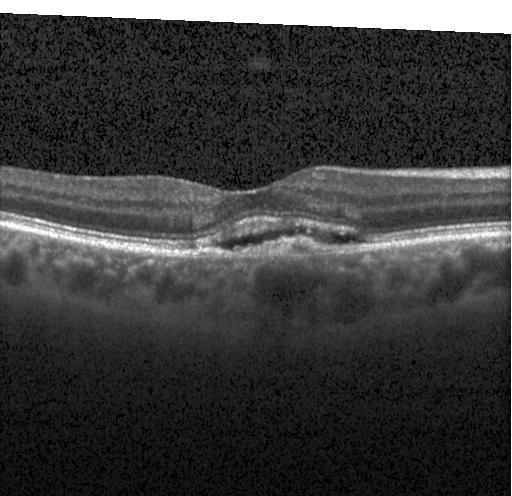 Heidelberg Spectralis OCT system, retinal OCT cross-section, through the macula, spectral-domain optical coherence tomography
Diagnosis: choroidal neovascularization (CNV).